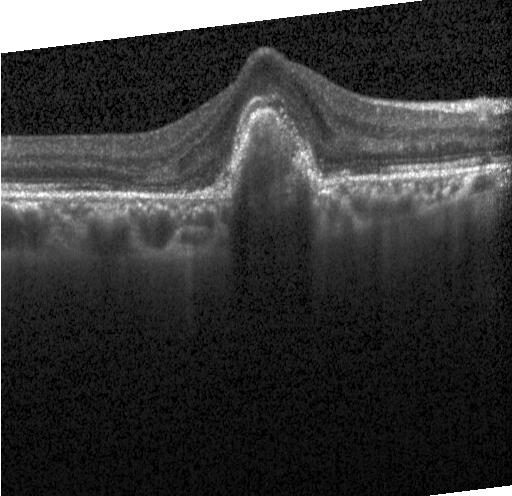
Macular OCT demonstrating a choroidal neovascular membrane.